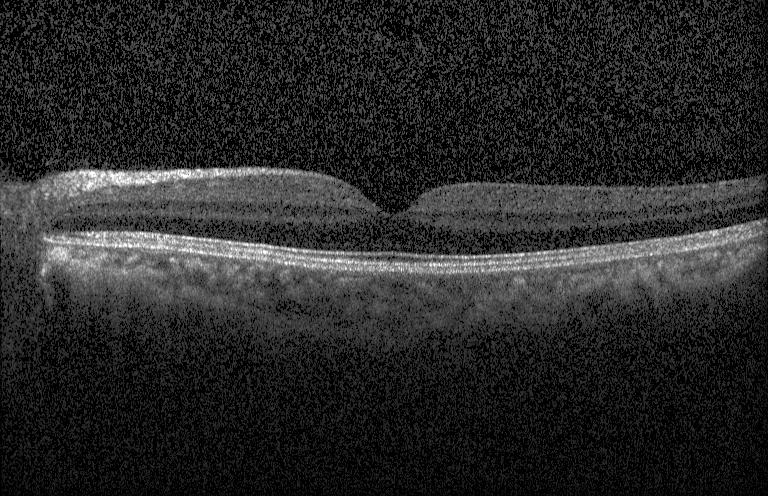 OCT B-scan. Spectral-domain OCT. Macular scan. Acquired on a Heidelberg Spectralis — Finding: no choroidal neovascularization, no diabetic macular edema, and no drusen.